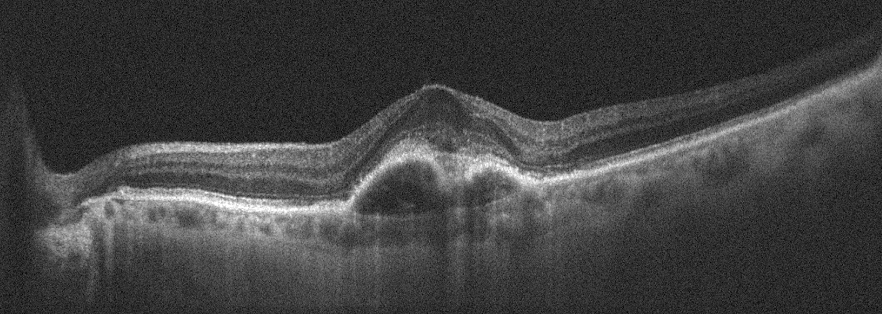

Optical coherence tomography B-scan; OS. This B-scan demonstrates age-related macular degeneration (AMD).